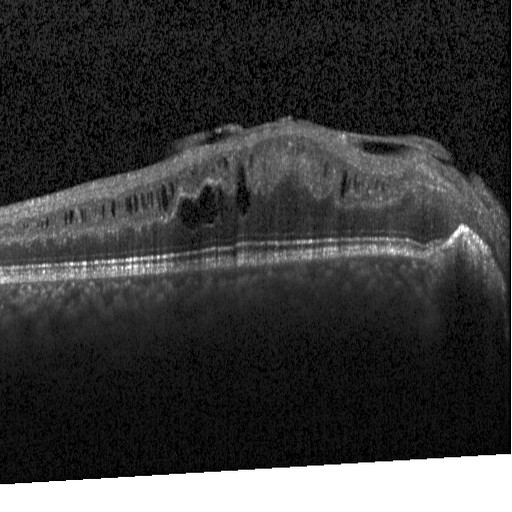 Instrument: Heidelberg Spectralis; OCT B-scan — Finding: DME.